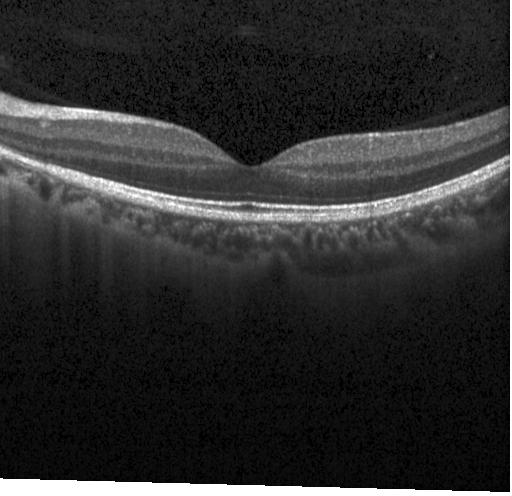
Retinal OCT cross-section showing no CNV, no DME, and no drusen.